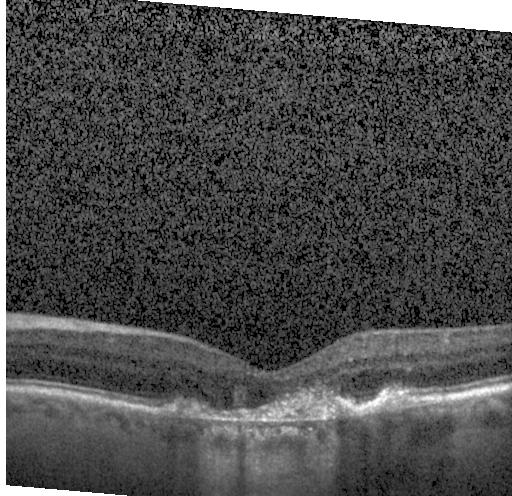 Centered on the fovea; instrument: Heidelberg Spectralis; spectral-domain OCT; optical coherence tomography B-scan. Dx: a choroidal neovascular membrane.